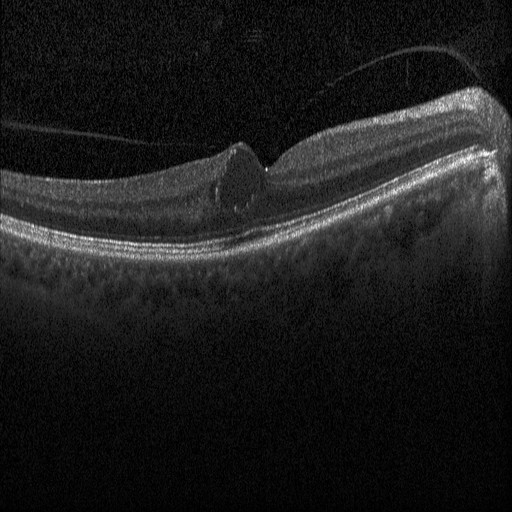
Impression: diabetic macular edema (DME).